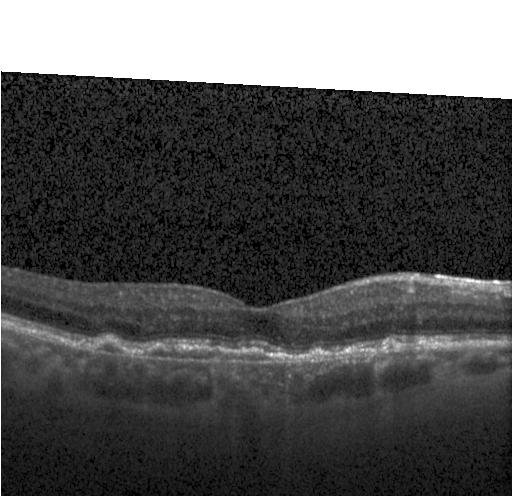

Macular OCT demonstrating CNV.